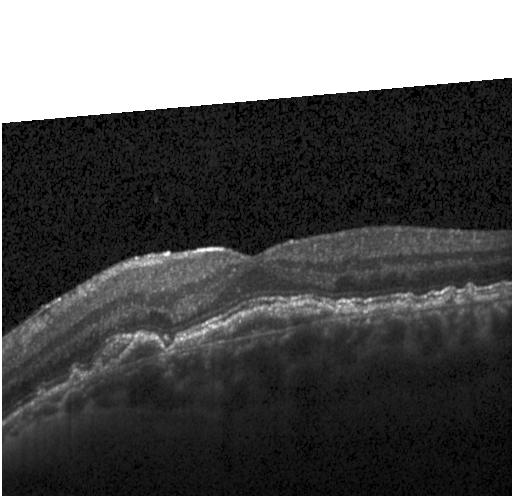
Through the macula · retinal OCT cross-section · spectral-domain optical coherence tomography. Finding: a choroidal neovascular membrane.